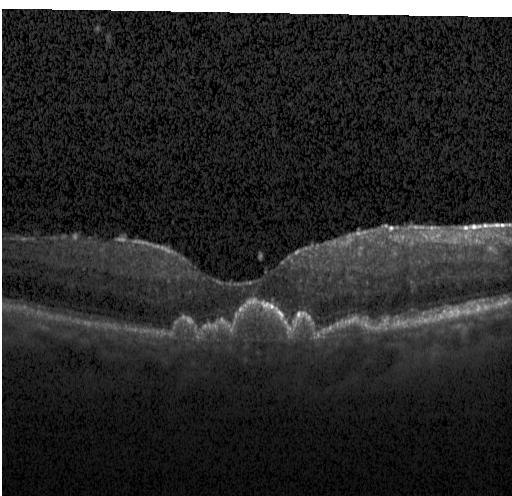
Heidelberg Spectralis OCT system · optical coherence tomography scan
The scan shows sub-RPE drusenoid deposits.